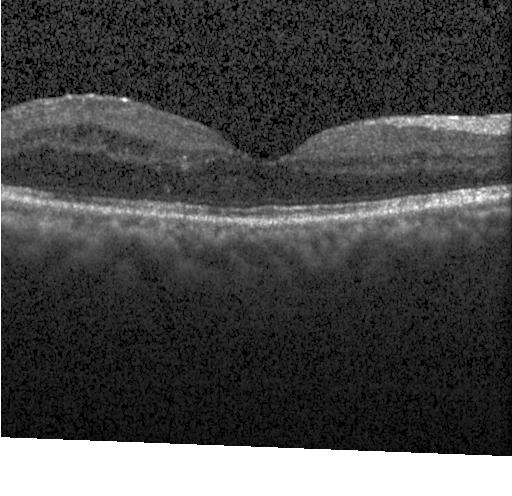

Optical coherence tomography B-scan. Impression: diabetic macular edema (DME).